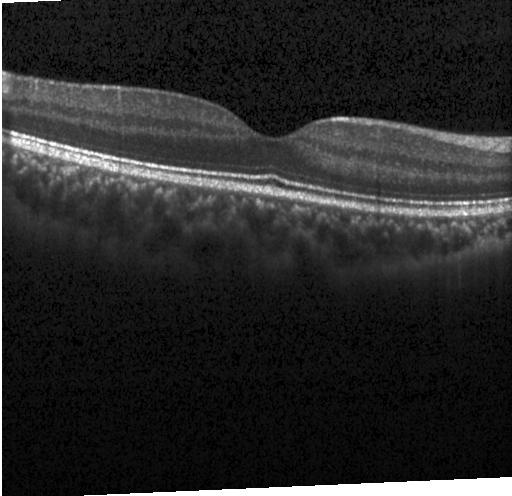
Acquired on a Heidelberg Spectralis. OCT line scan. SD-OCT. Fovea-centered.
Impression: no choroidal neovascularization, diabetic macular edema, or drusen.